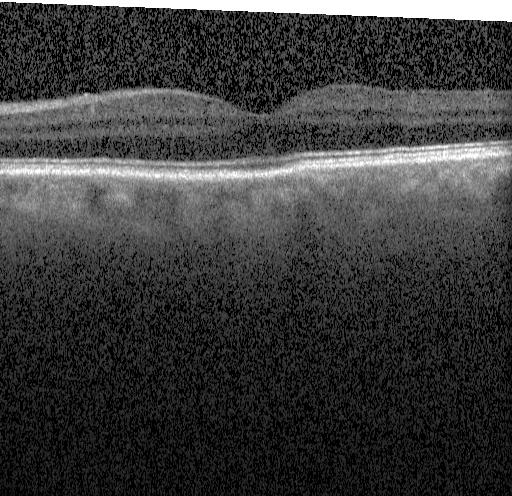 Macular OCT demonstrating no evidence of CNV, DME, or drusen.